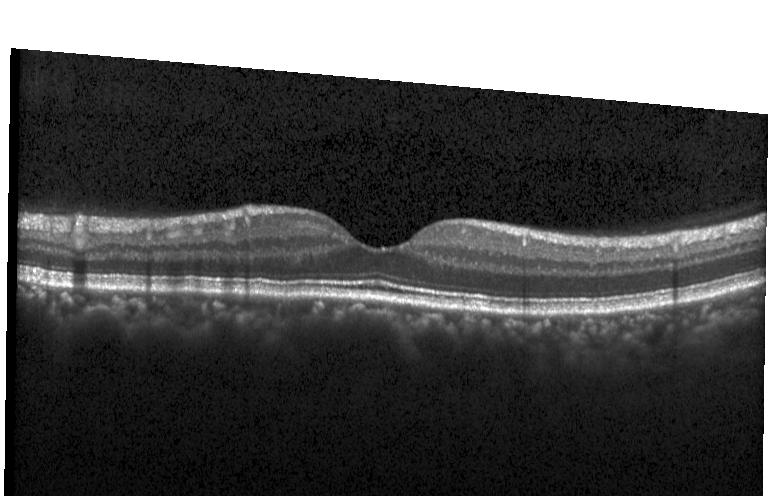

Retinal OCT B-scan; SD-OCT
Impression: no choroidal neovascularization, diabetic macular edema, or drusen.